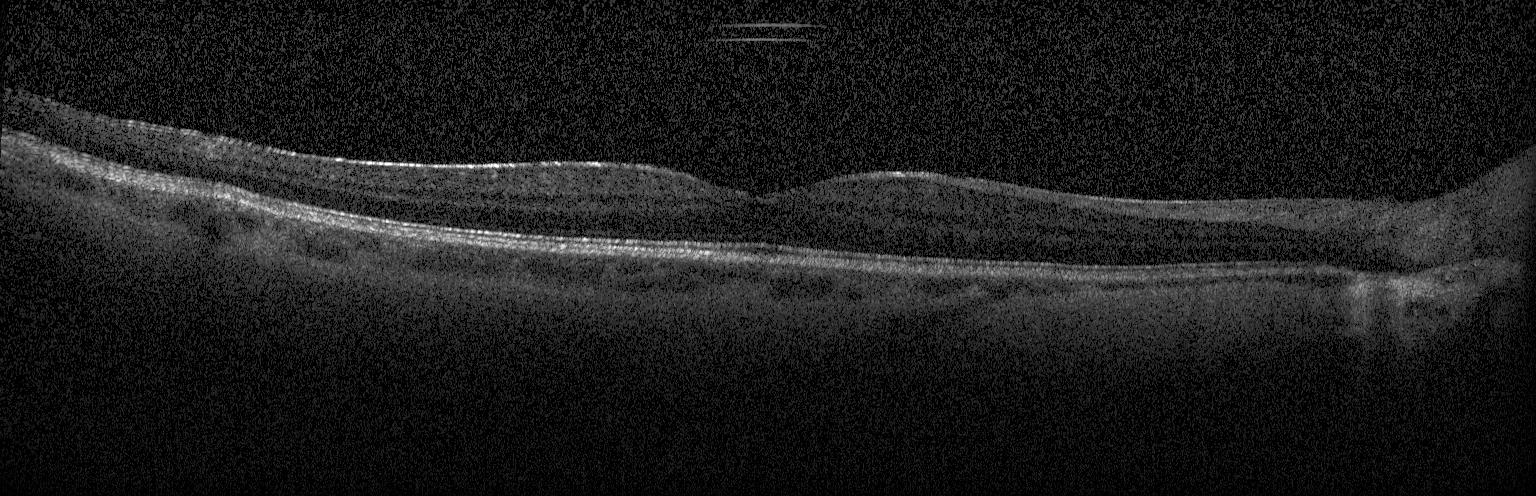

No evidence of choroidal neovascularization, diabetic macular edema, or drusen.